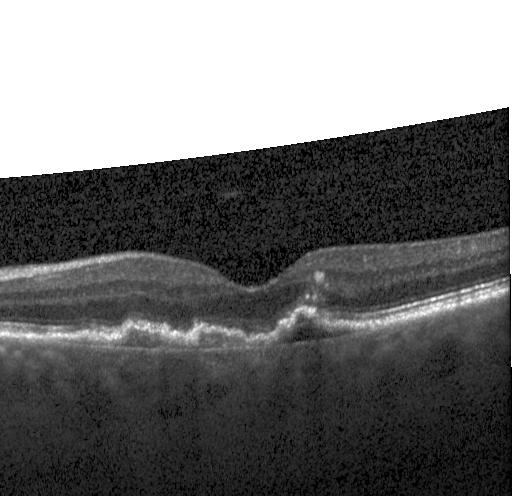
Dx: CNV.